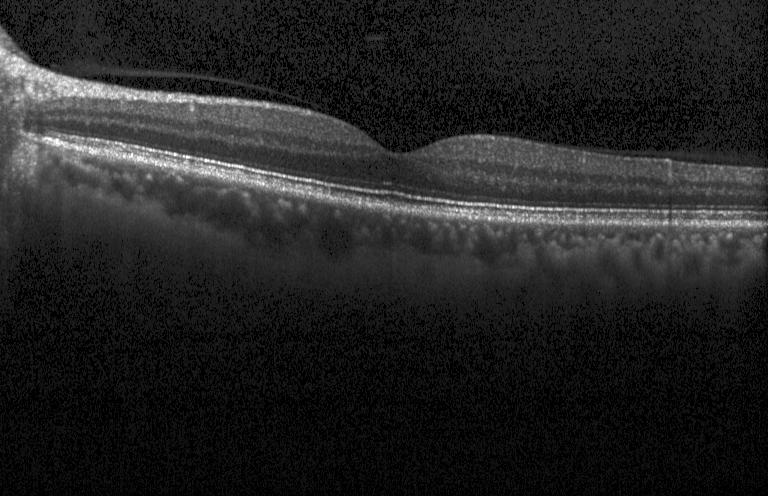
OCT line scan — Dx: neither choroidal neovascularization, diabetic macular edema, nor drusen.